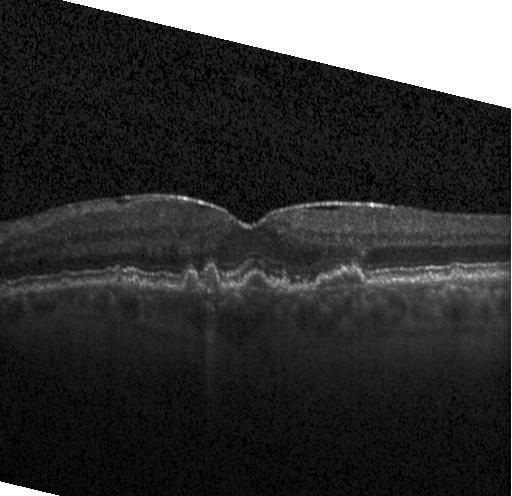

OCT B-scan, fovea-centered, acquired on a Heidelberg Spectralis, SD-OCT
Impression: drusen.